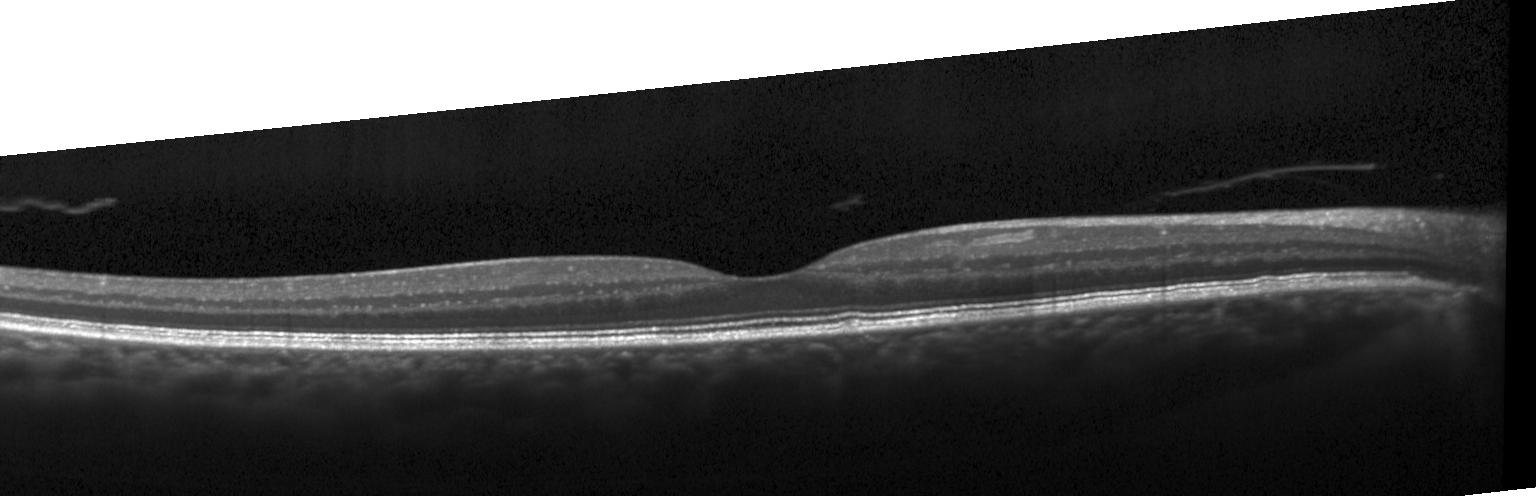
Diagnosis: neither choroidal neovascularization, diabetic macular edema, nor drusen.